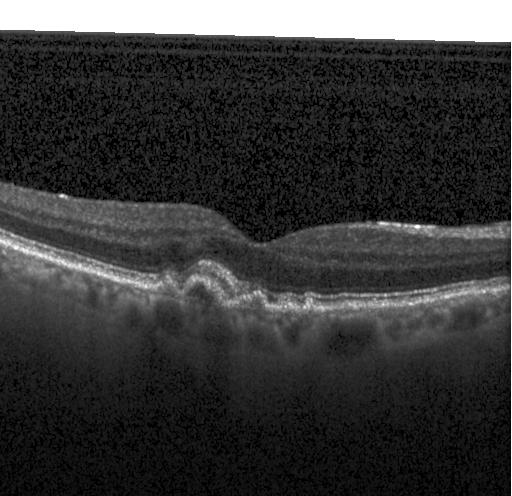 SD-OCT, retinal OCT B-scan, macular scan, Heidelberg Spectralis — Dx: CNV.